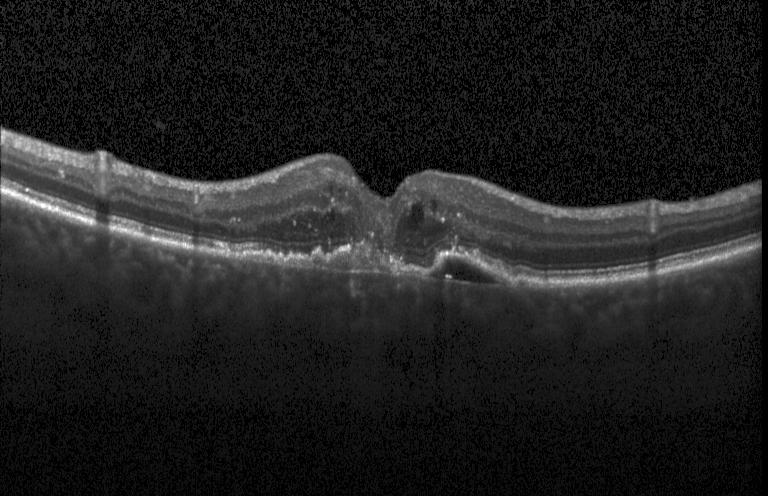

OCT B-scan showing choroidal neovascularization (CNV).